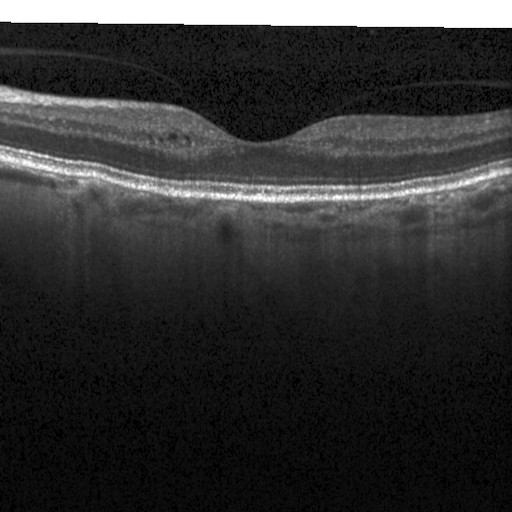 Diagnosis: DME.